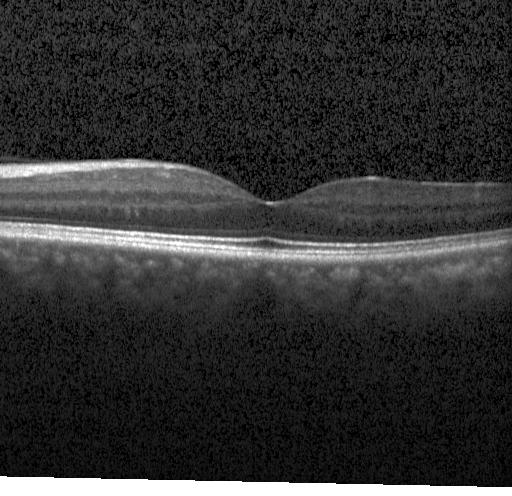

Heidelberg Spectralis. Optical coherence tomography scan. Spectral-domain OCT. Centered on the fovea.
OCT finding: neither choroidal neovascularization, diabetic macular edema, nor drusen.